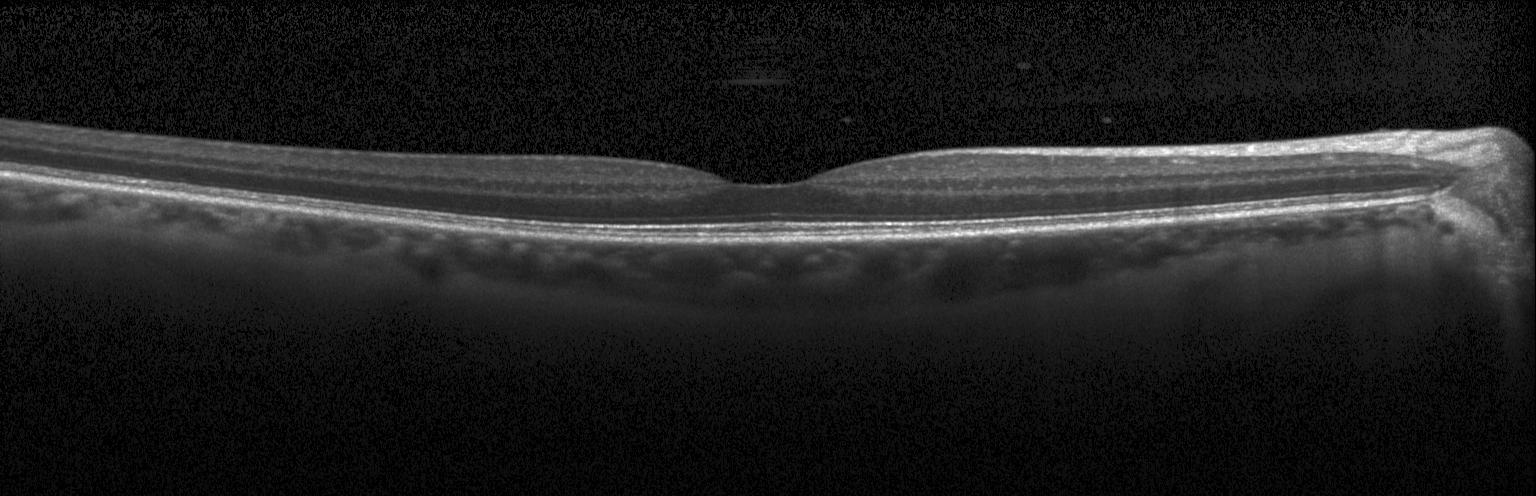 Horizontal scan through the fovea, spectral-domain optical coherence tomography, OCT B-scan — The scan shows neither CNV, DME, nor drusen.